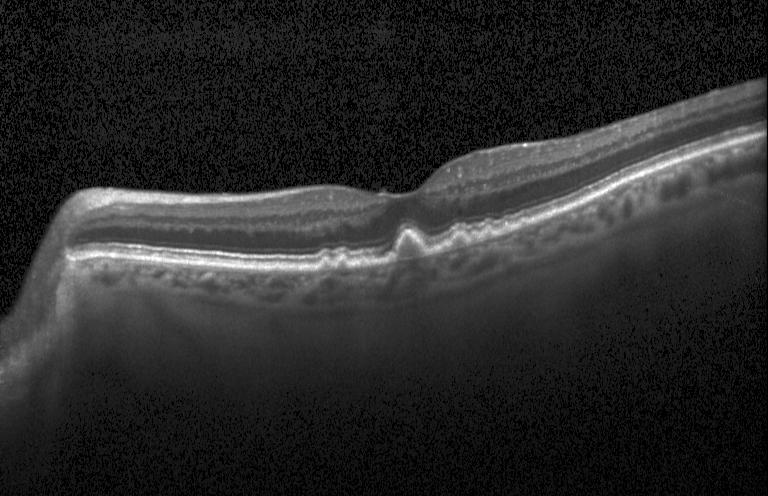 OCT B-scan, spectral-domain OCT — Dx: sub-RPE drusenoid deposits.